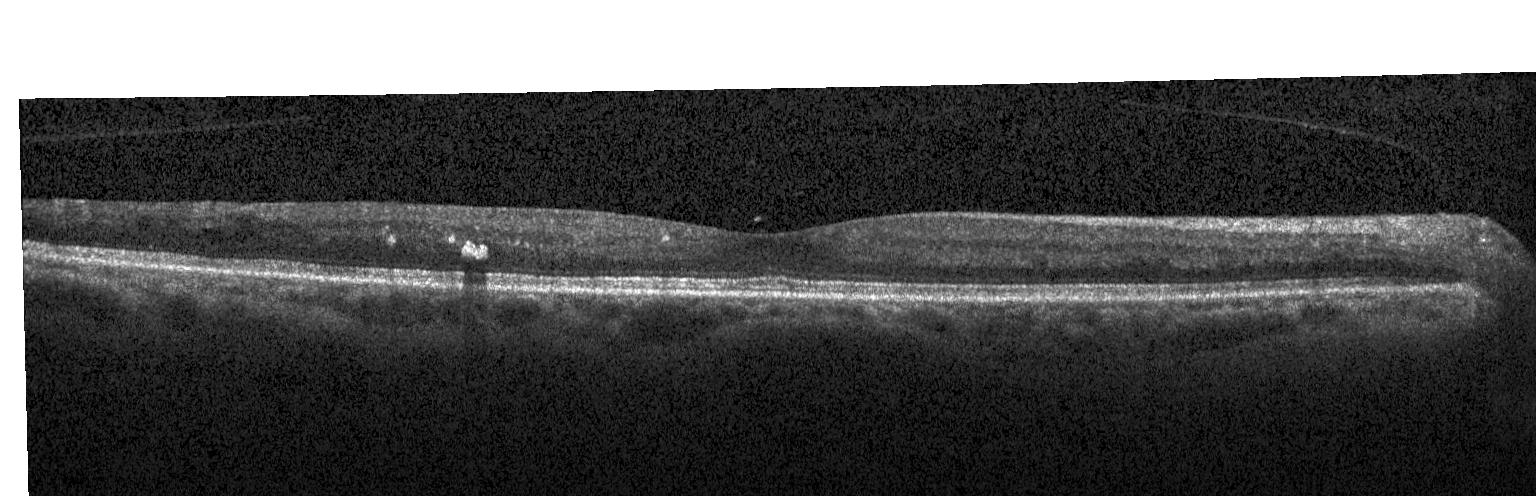
OCT B-scan
This B-scan demonstrates DME.